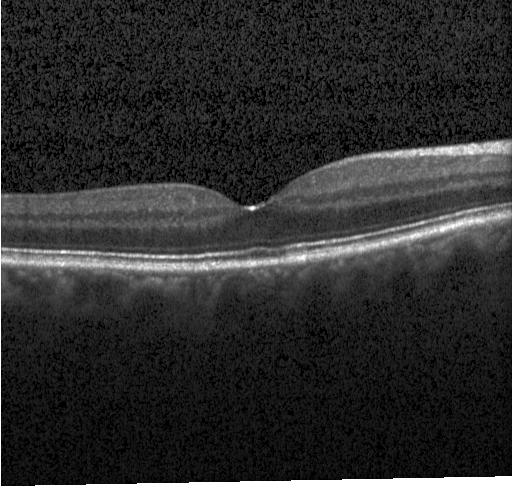 Heidelberg Spectralis · OCT B-scan. Dx: no choroidal neovascularization, diabetic macular edema, or drusen.